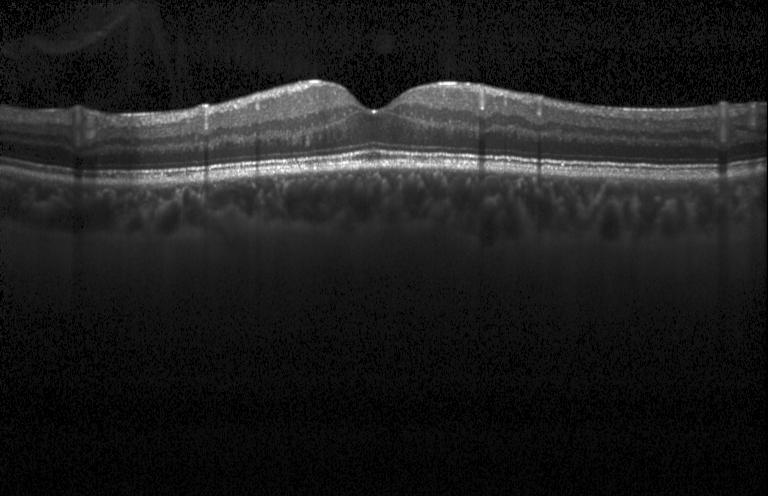

Retinal OCT cross-section · fovea-centered · spectral-domain optical coherence tomography.
Macular OCT: no CNV, no DME, and no drusen.